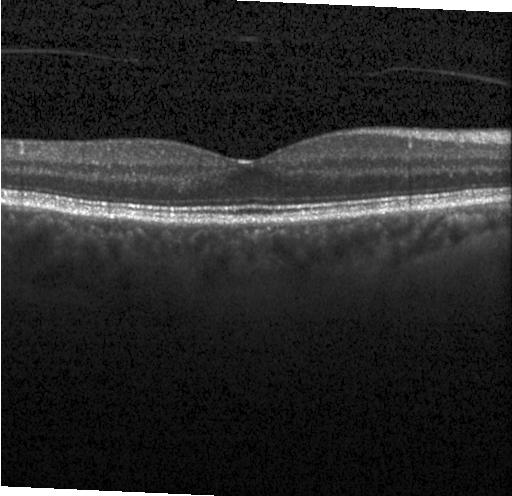
Finding: no evidence of CNV, DME, or drusen.